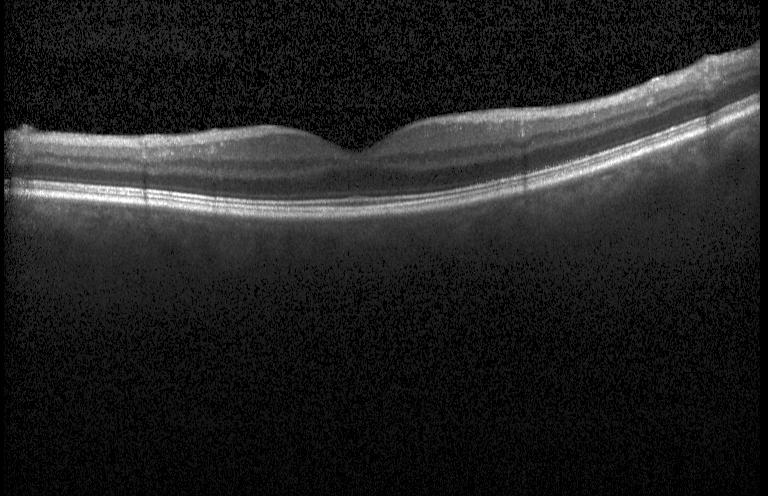
Assessment: no choroidal neovascularization, no diabetic macular edema, and no drusen.